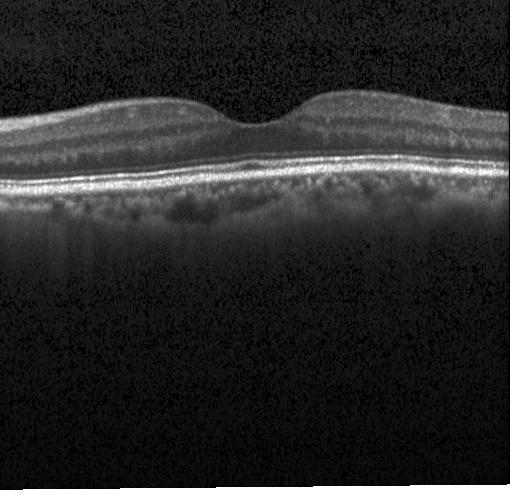

Diagnosis: no choroidal neovascularization, diabetic macular edema, or drusen.